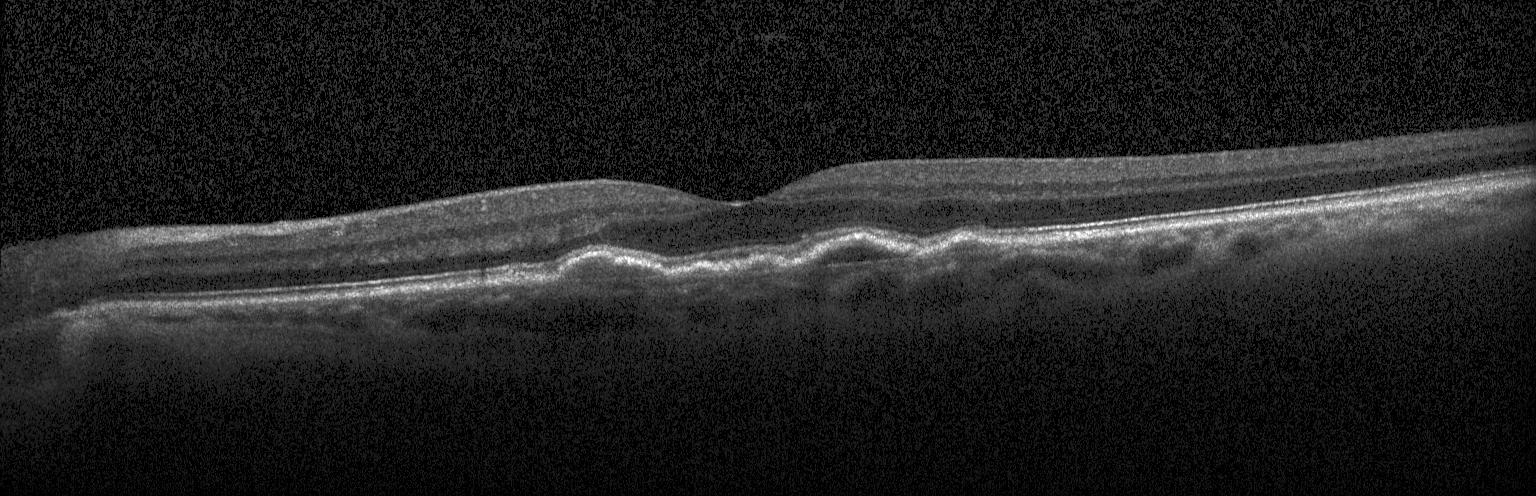 Spectral-domain optical coherence tomography. OCT B-scan. Instrument: Heidelberg Spectralis — Finding: multiple drusen.